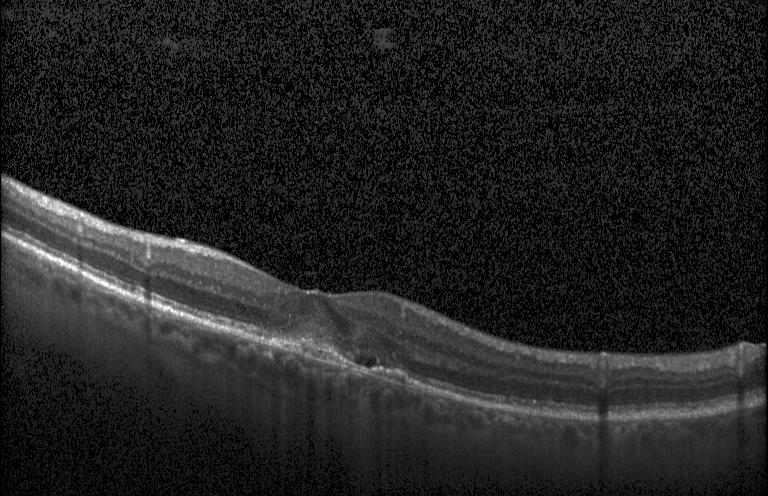

Optical coherence tomography B-scan · spectral-domain optical coherence tomography — This B-scan demonstrates CNV.